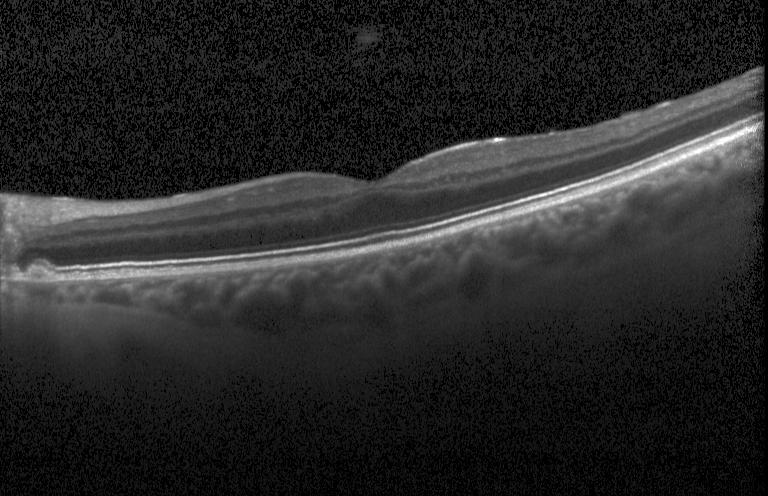

Macular OCT: no CNV, no DME, and no drusen.